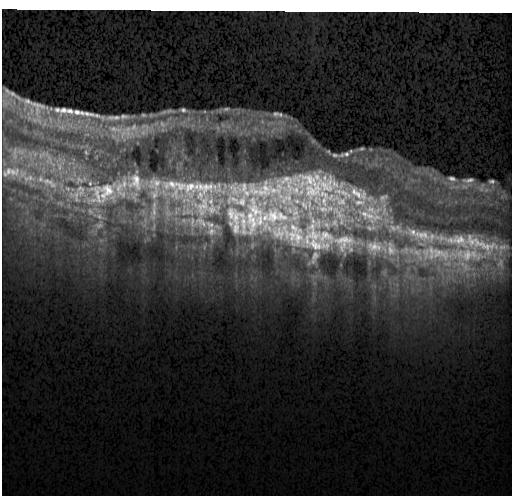

Acquired on a Heidelberg Spectralis · OCT B-scan · macular scan · SD-OCT — Finding: choroidal neovascularization (CNV).